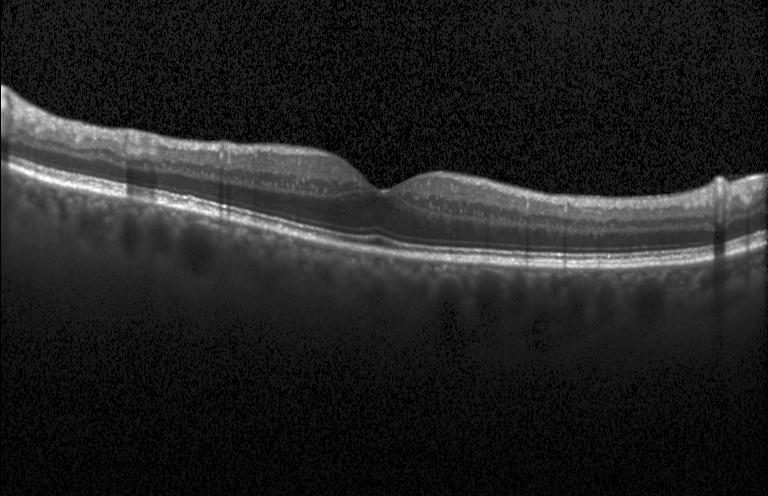

This B-scan demonstrates no evidence of CNV, DME, or drusen.